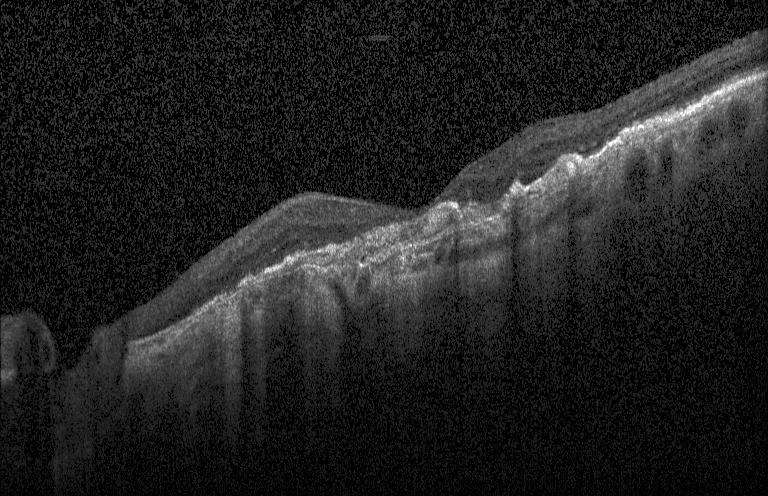 OCT B-scan showing choroidal neovascularization.